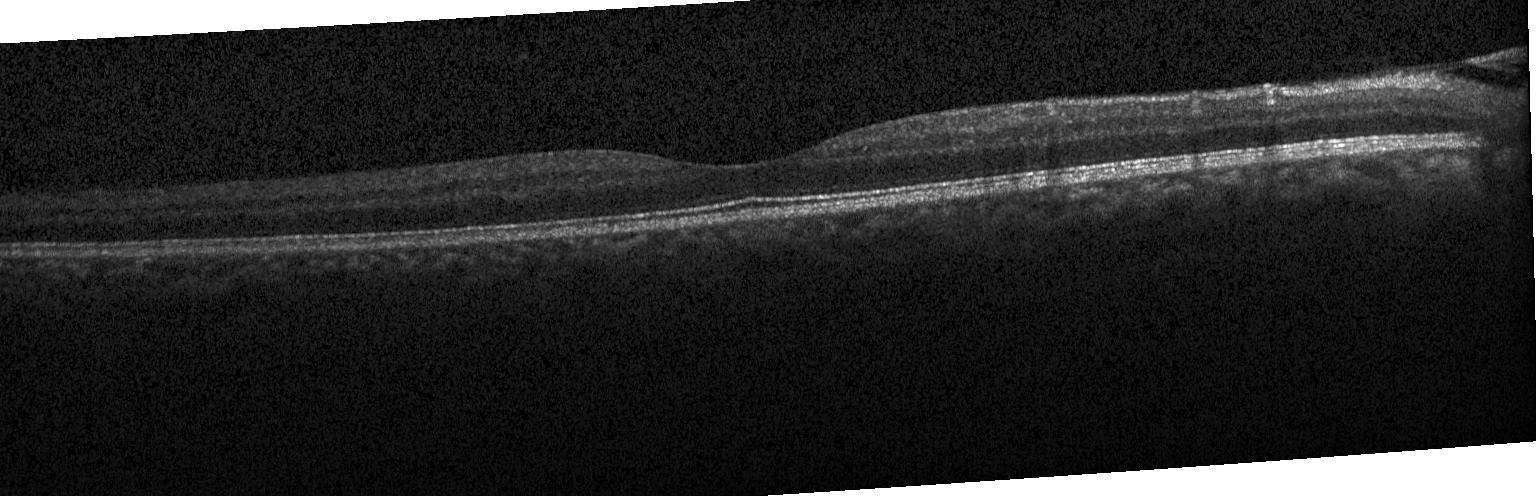

OCT line scan. Acquired on a Heidelberg Spectralis. SD-OCT.
Impression: no evidence of choroidal neovascularization, diabetic macular edema, or drusen.